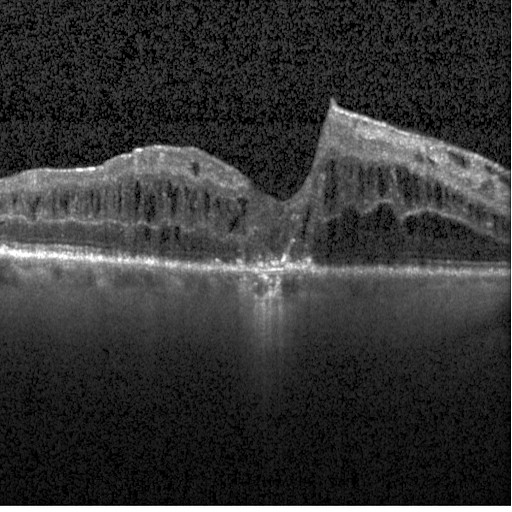 OCT line scan; fovea-centered; spectral-domain optical coherence tomography.
This B-scan demonstrates diabetic macular edema.